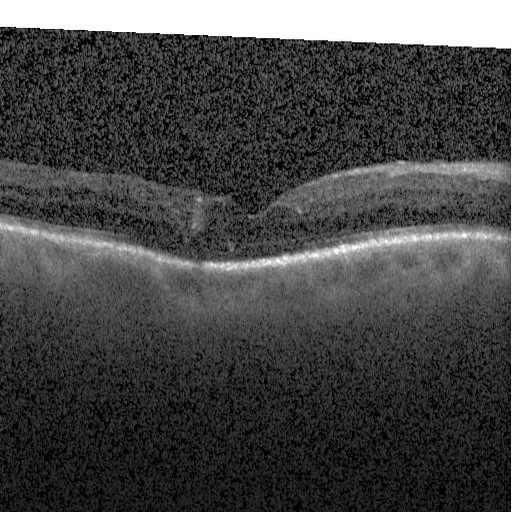
Finding: DME.